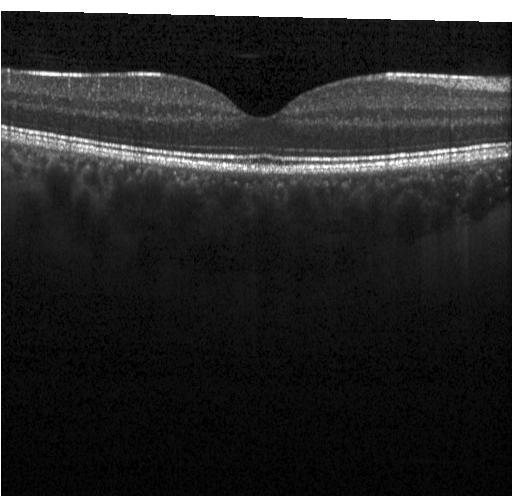 Retinal OCT B-scan
Finding: no choroidal neovascularization, no diabetic macular edema, and no drusen.